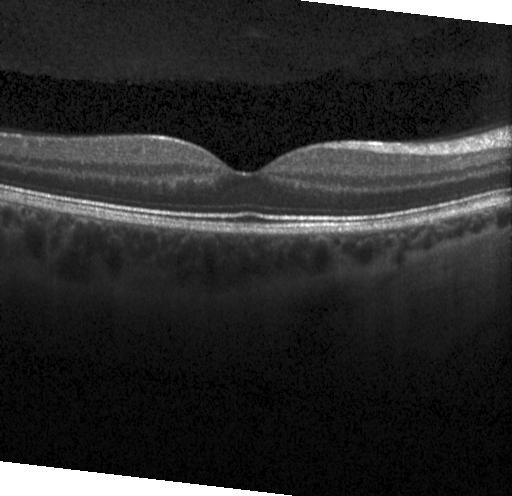
Dx: neither CNV, DME, nor drusen.